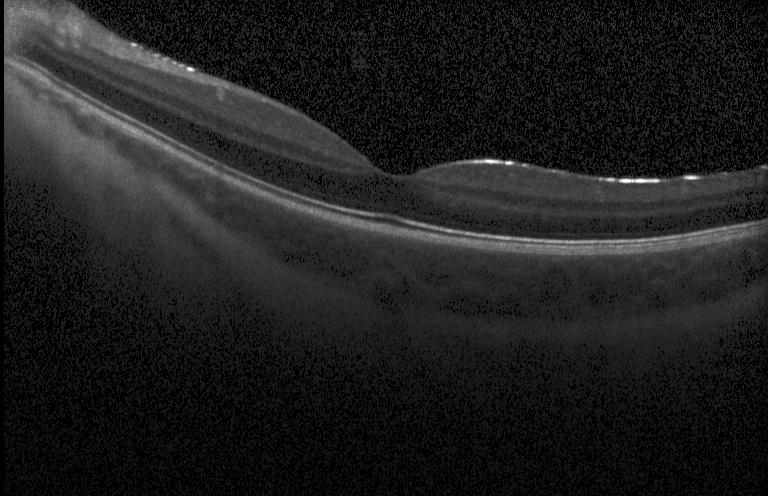

Dx: no choroidal neovascularization, diabetic macular edema, or drusen.